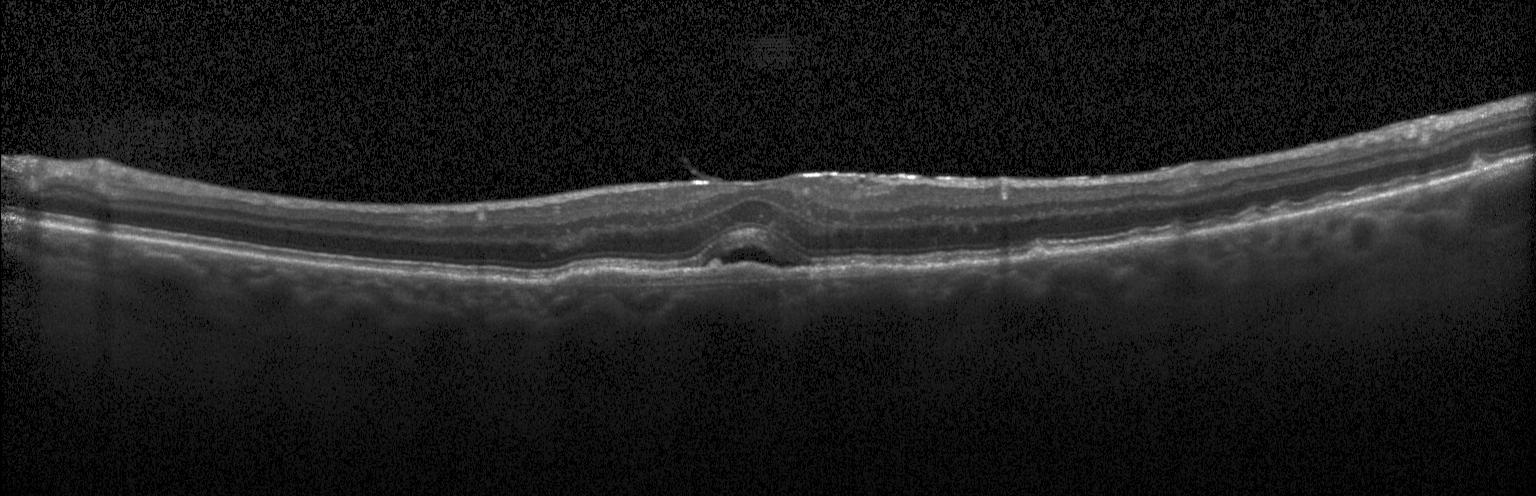

Dx: a choroidal neovascular membrane.